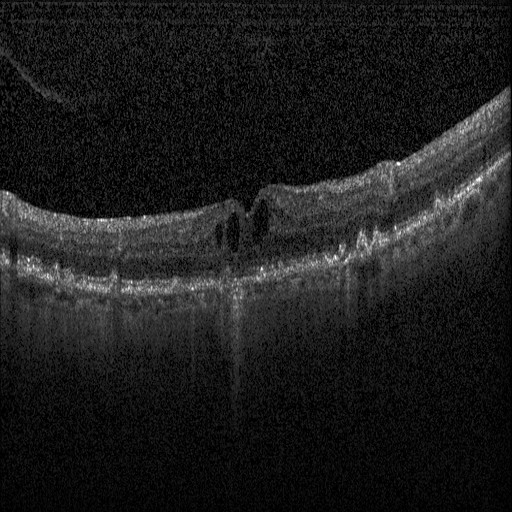

OCT line scan. SD-OCT. Impression: diabetic macular edema.